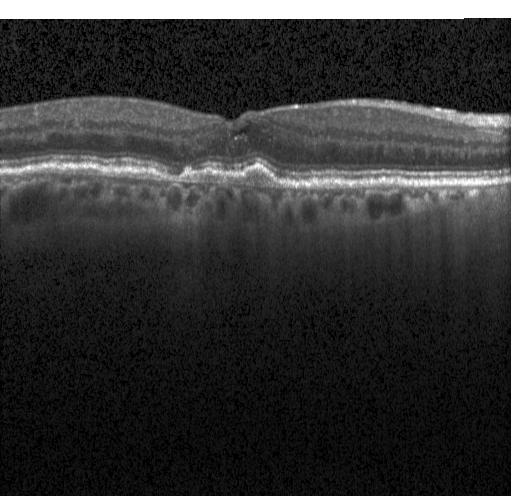

Fovea-centered · spectral-domain optical coherence tomography · retinal OCT cross-section
Diagnosis: a choroidal neovascular membrane.